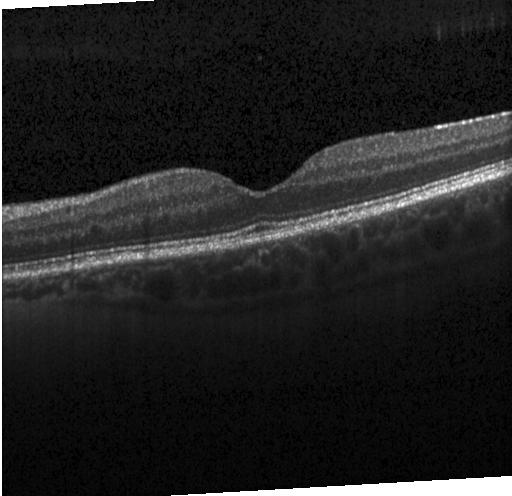
Centered on the fovea · retinal OCT cross-section.
Impression: no choroidal neovascularization, no diabetic macular edema, and no drusen.